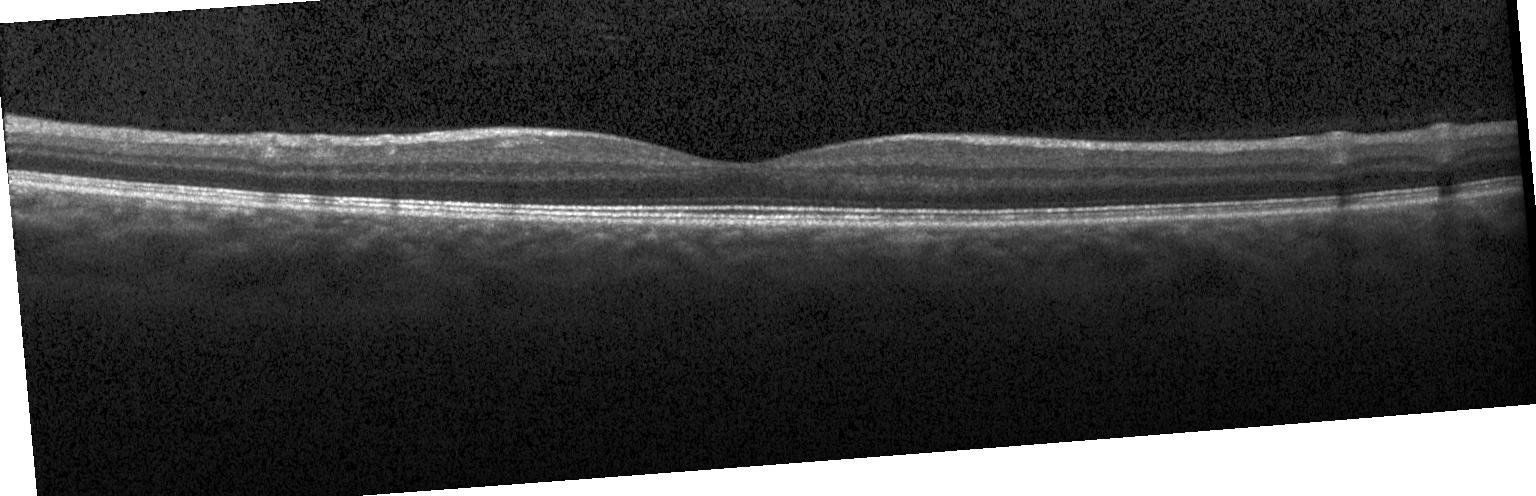
Spectral-domain OCT; retinal OCT B-scan.
Diagnosis: no CNV, DME, or drusen.